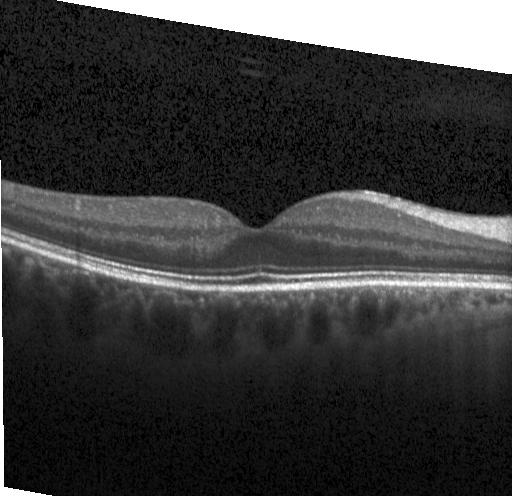

OCT line scan, spectral-domain OCT — This B-scan demonstrates no evidence of choroidal neovascularization, diabetic macular edema, or drusen.